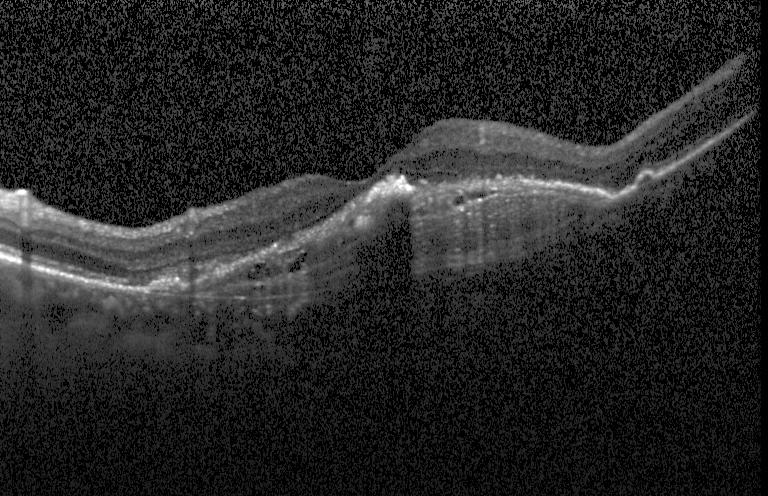 OCT B-scan
The scan shows a choroidal neovascular membrane.